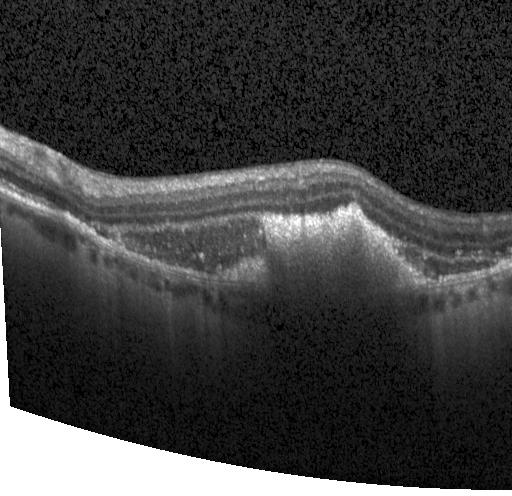

Optical coherence tomography B-scan; spectral-domain optical coherence tomography — Assessment: a choroidal neovascular membrane.